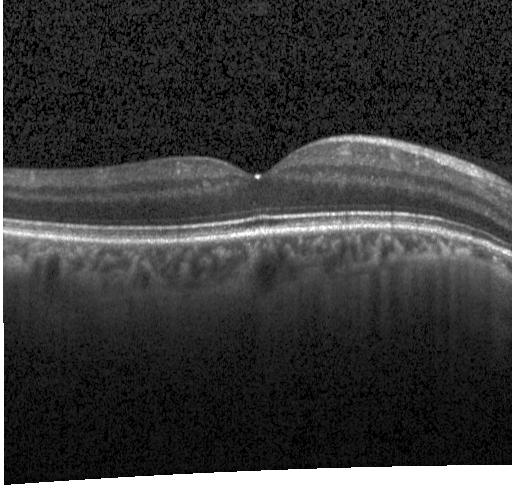
Spectral-domain OCT, acquired on a Heidelberg Spectralis, optical coherence tomography scan. Diagnosis: neither choroidal neovascularization, diabetic macular edema, nor drusen.